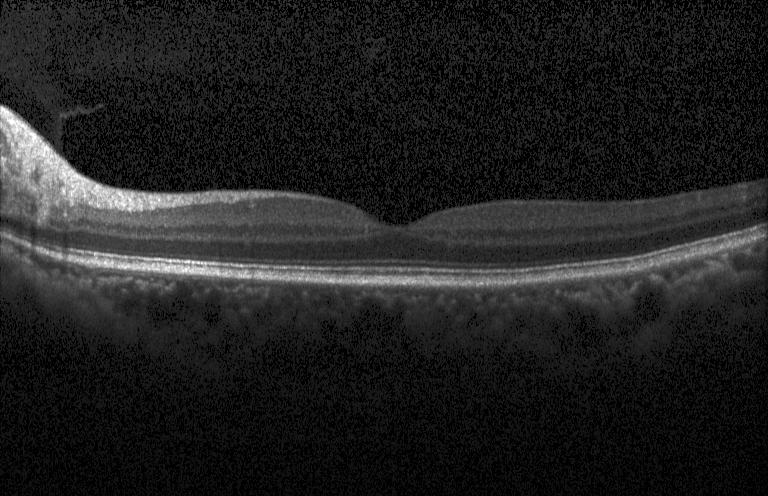 Heidelberg Spectralis OCT system, retinal OCT cross-section
Impression: no evidence of CNV, DME, or drusen.